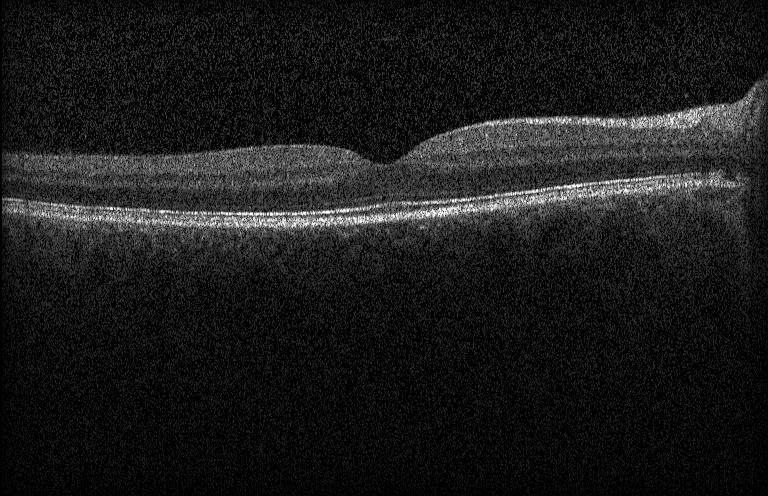
OCT B-scan
Macular OCT: no evidence of choroidal neovascularization, diabetic macular edema, or drusen.